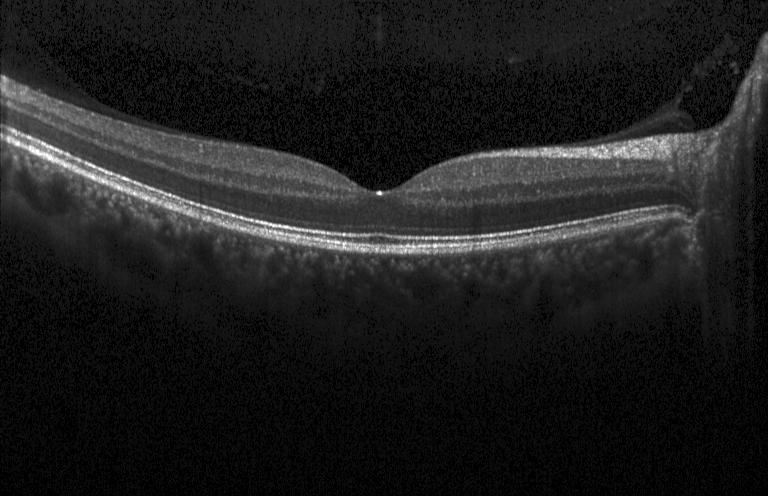
OCT finding: neither choroidal neovascularization, diabetic macular edema, nor drusen.